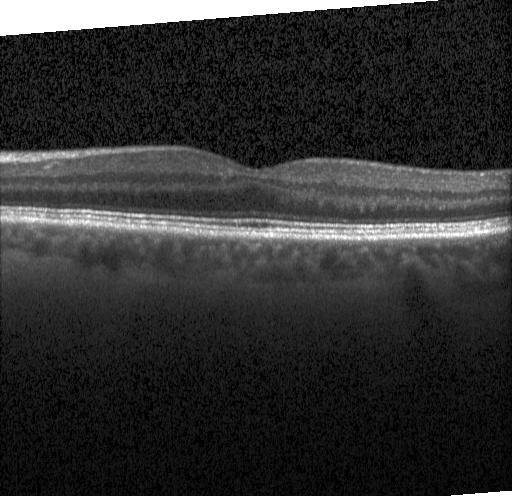
OCT scan showing neither choroidal neovascularization, diabetic macular edema, nor drusen.